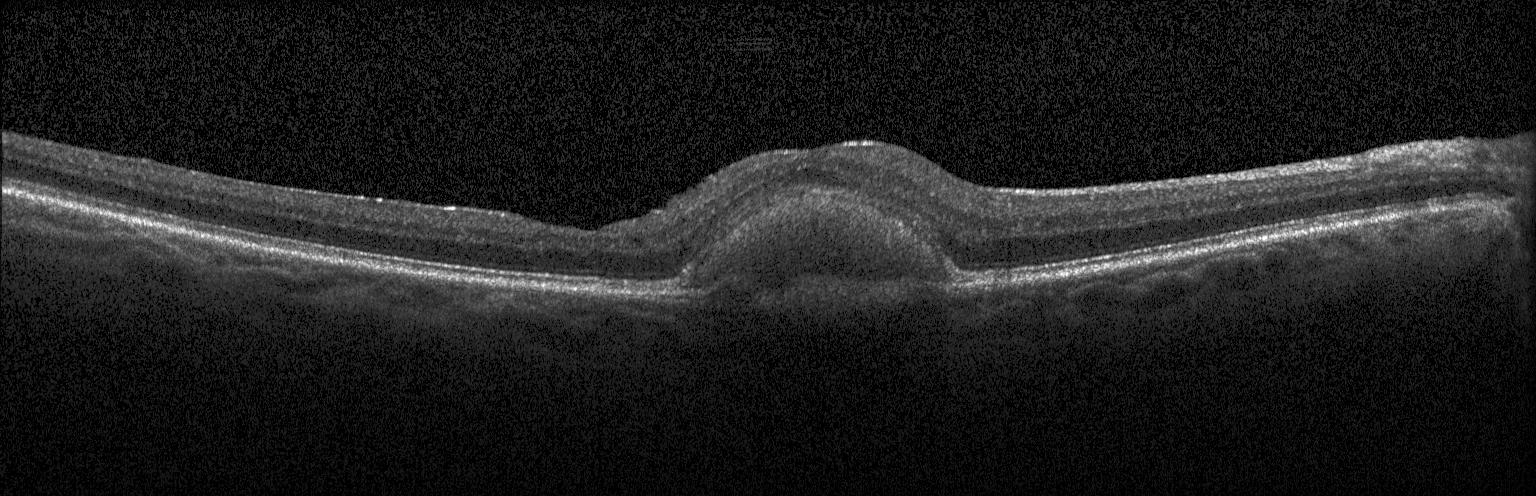 Finding: choroidal neovascularization (CNV).